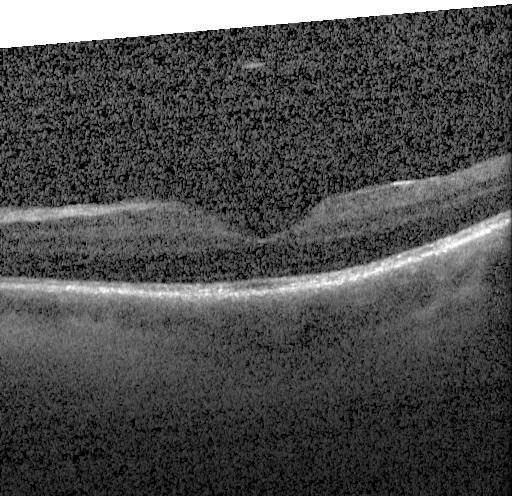 Dx: no evidence of CNV, DME, or drusen.